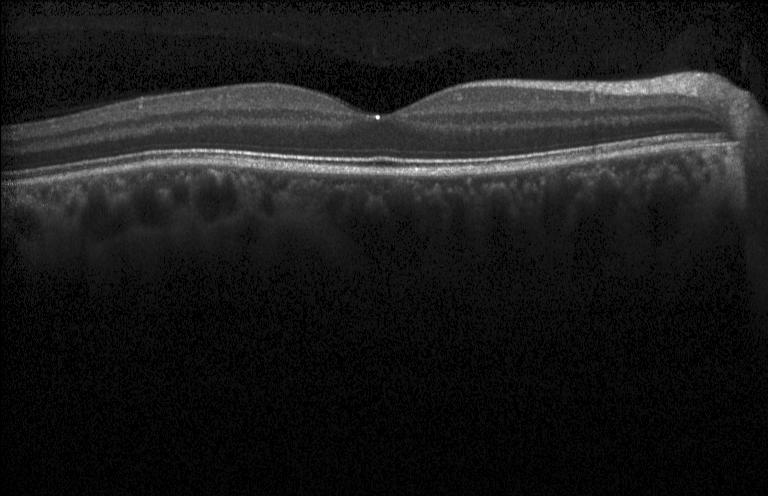
Optical coherence tomography scan. The scan shows no evidence of choroidal neovascularization, diabetic macular edema, or drusen.